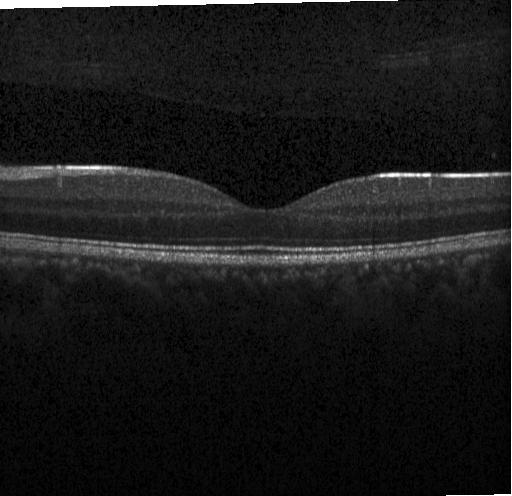

Retinal OCT cross-section; centered on the fovea — The scan shows neither choroidal neovascularization, diabetic macular edema, nor drusen.